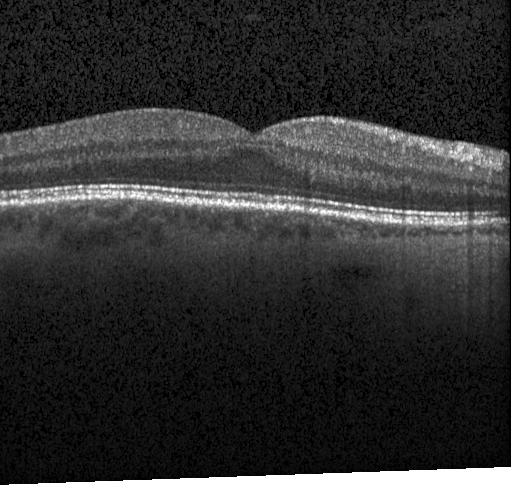 Optical coherence tomography B-scan
Finding: no evidence of CNV, DME, or drusen.